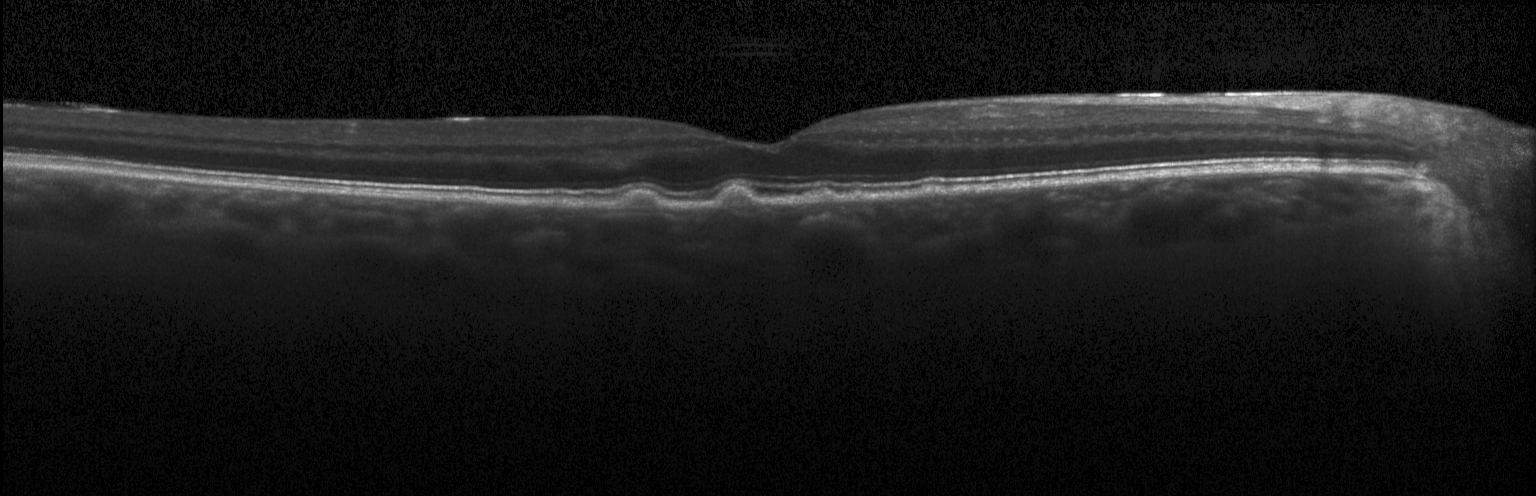
SD-OCT. Heidelberg Spectralis OCT system. Optical coherence tomography B-scan.
OCT finding: multiple drusen.